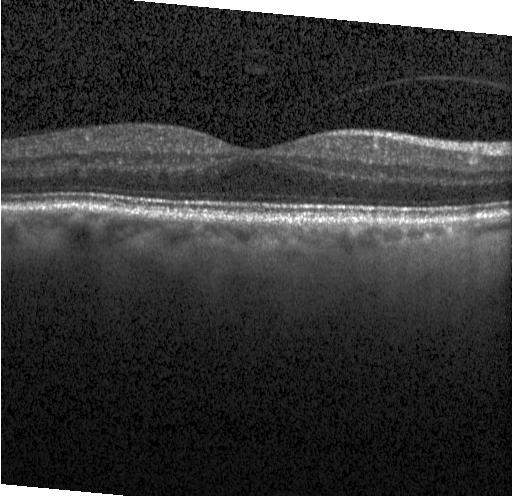
Optical coherence tomography B-scan — The scan shows no choroidal neovascularization, diabetic macular edema, or drusen.